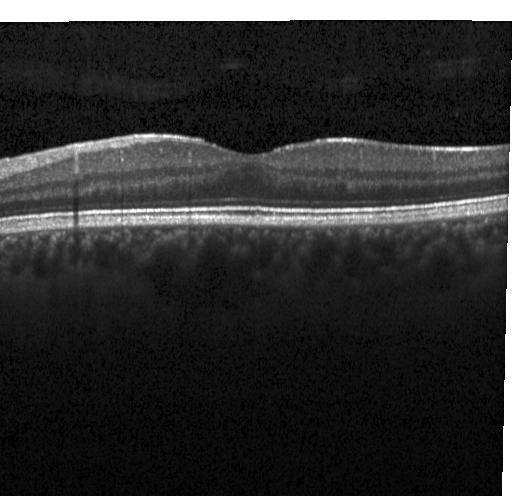 OCT B-scan showing no evidence of CNV, DME, or drusen.